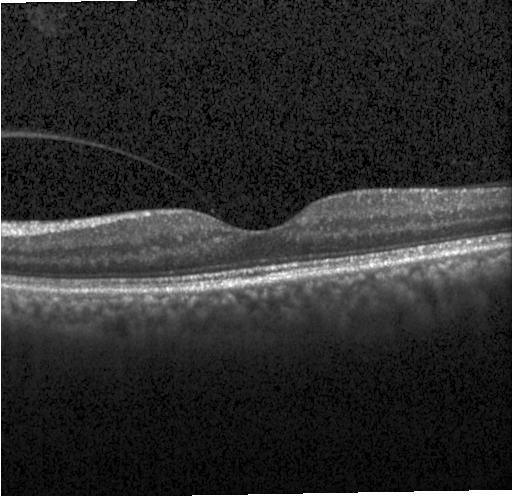 Heidelberg Spectralis. OCT B-scan.
This B-scan demonstrates neither choroidal neovascularization, diabetic macular edema, nor drusen.